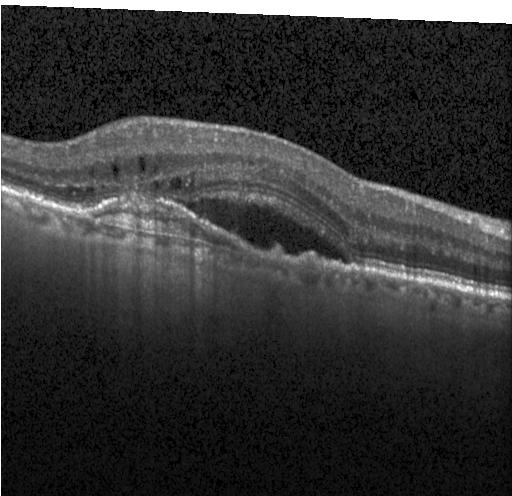

Impression: CNV.